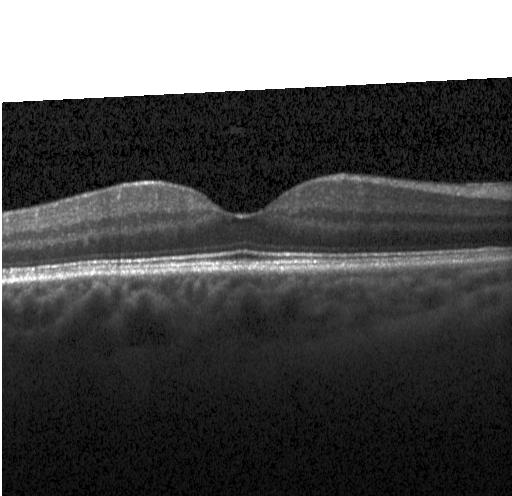

Optical coherence tomography B-scan. Dx: no choroidal neovascularization, no diabetic macular edema, and no drusen.